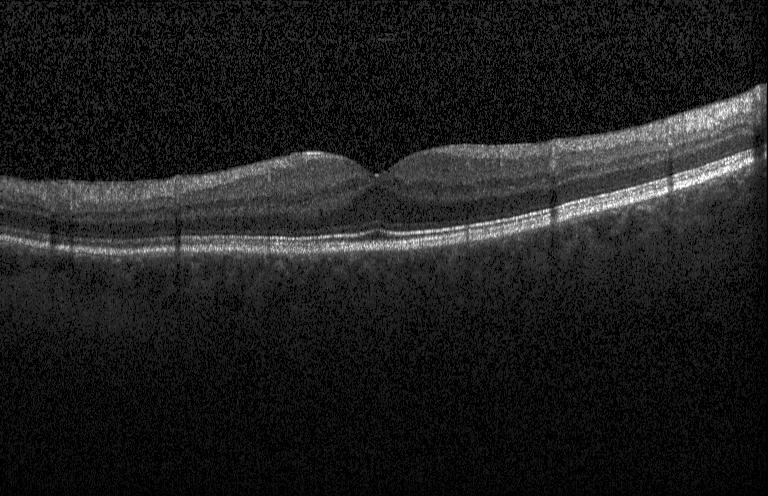 OCT line scan. Horizontal scan through the fovea — Assessment: no CNV, no DME, and no drusen.